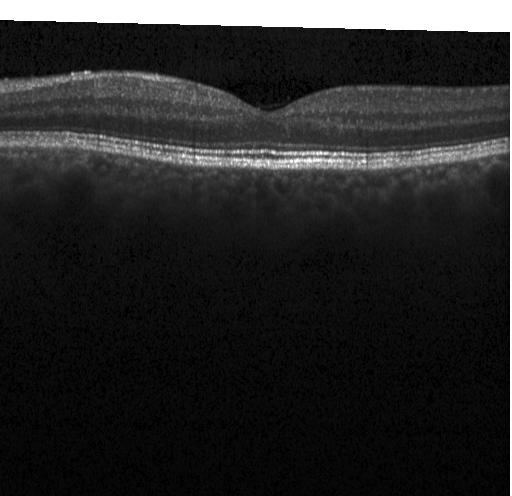

Centered on the fovea. OCT line scan. Spectral-domain optical coherence tomography. Acquired on a Heidelberg Spectralis. Macular OCT: no CNV, DME, or drusen.